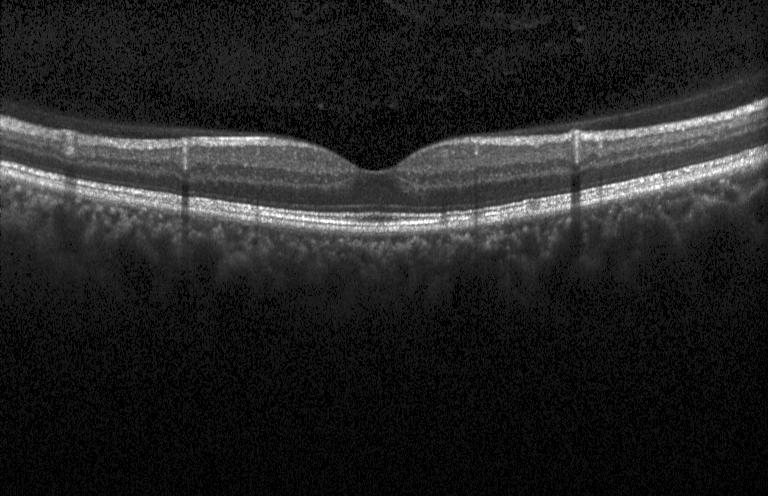 Horizontal scan through the fovea; retinal OCT B-scan
Impression: no choroidal neovascularization, no diabetic macular edema, and no drusen.